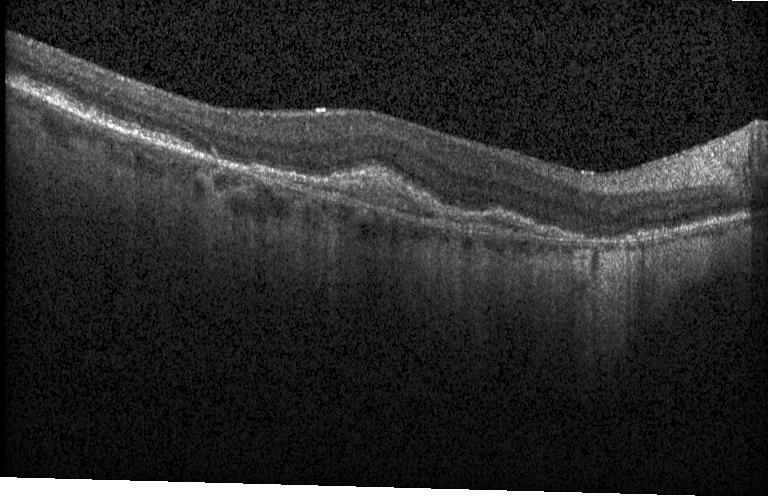 Spectral-domain OCT. Centered on the fovea. OCT line scan. Heidelberg Spectralis OCT system
OCT finding: choroidal neovascularization (CNV).